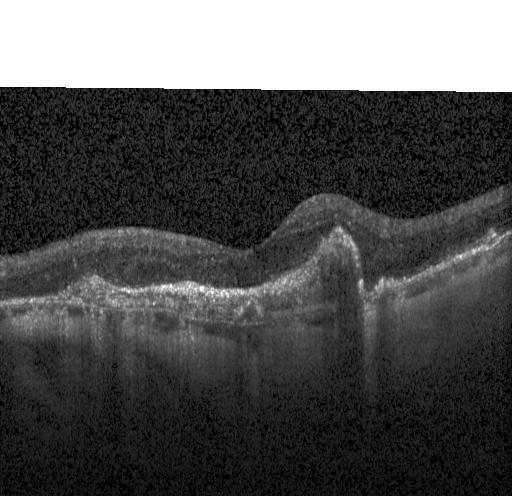 This B-scan demonstrates a choroidal neovascular membrane.